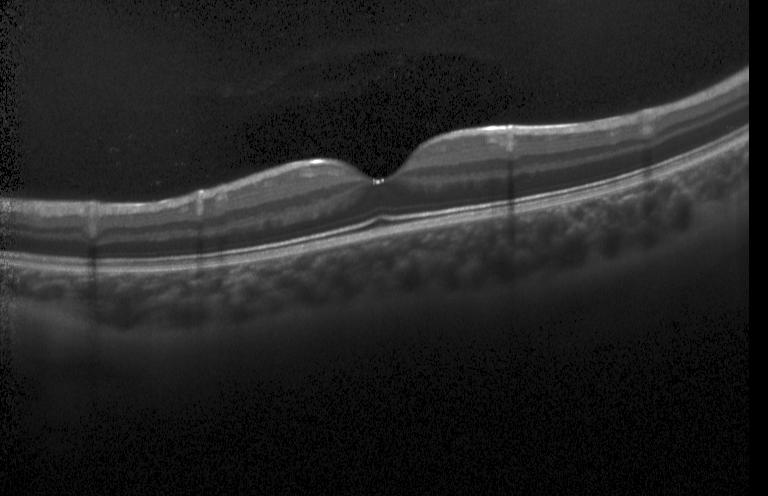

Through the macula · OCT line scan · Heidelberg Spectralis OCT system. Finding: no evidence of CNV, DME, or drusen.